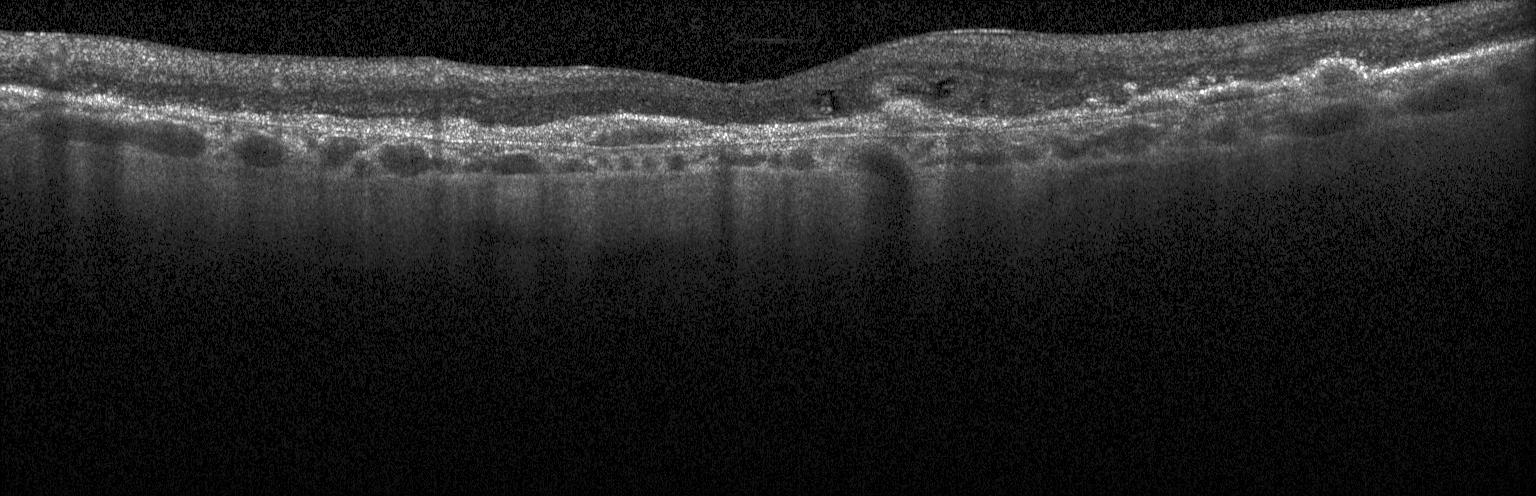
A choroidal neovascular membrane.